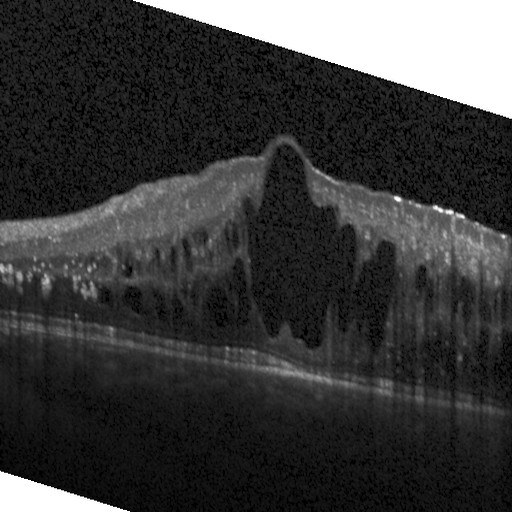 Heidelberg Spectralis OCT system, retinal OCT B-scan
This B-scan demonstrates diabetic macular edema.